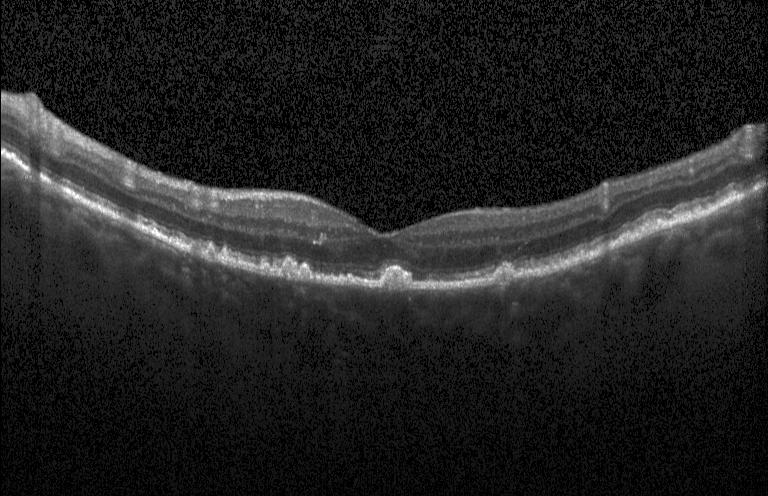 Dx: choroidal neovascularization.